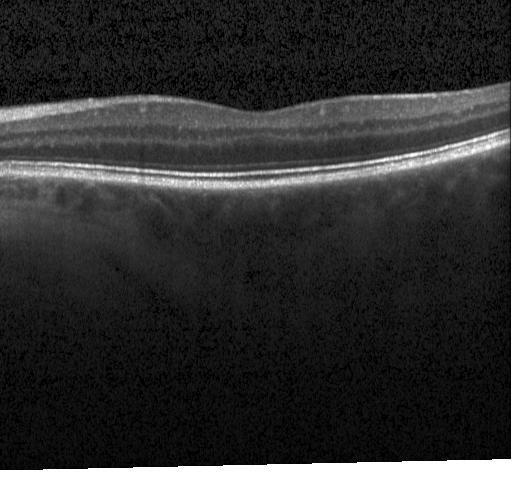

Acquired on a Heidelberg Spectralis · through the macula · retinal OCT cross-section.
Diagnosis: no CNV, DME, or drusen.